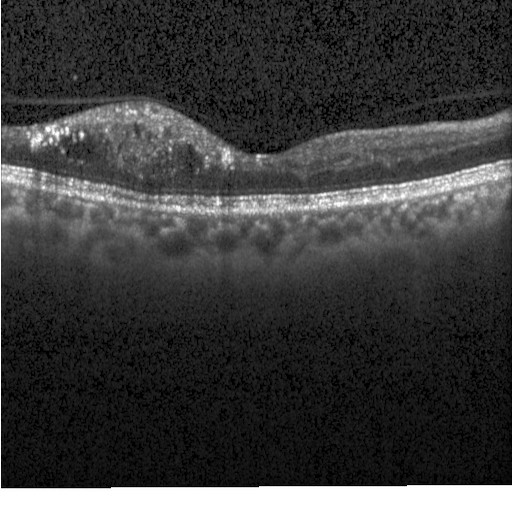

Macular OCT: diabetic macular edema (DME).